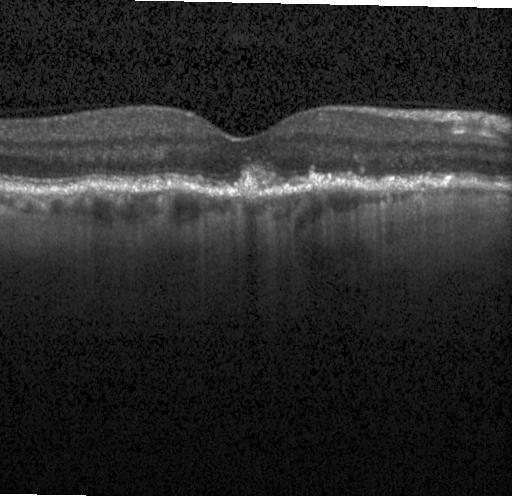

Horizontal scan through the fovea; instrument: Heidelberg Spectralis; optical coherence tomography B-scan; SD-OCT
Sub-RPE drusenoid deposits.